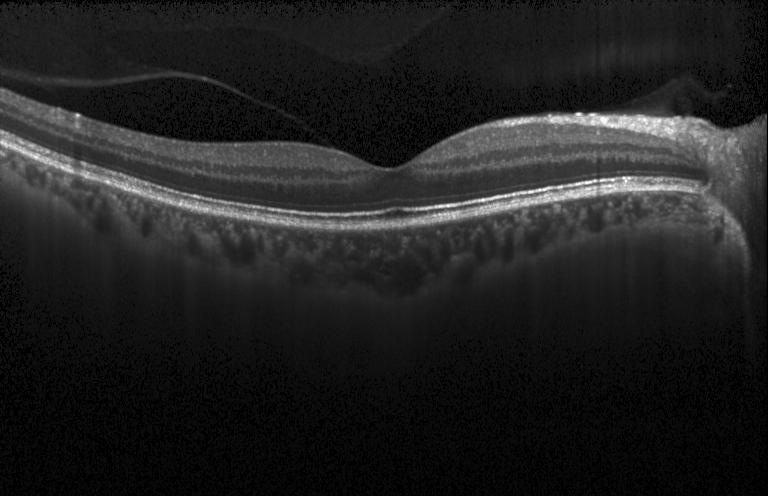

Instrument: Heidelberg Spectralis · OCT B-scan · fovea-centered — Finding: no evidence of choroidal neovascularization, diabetic macular edema, or drusen.